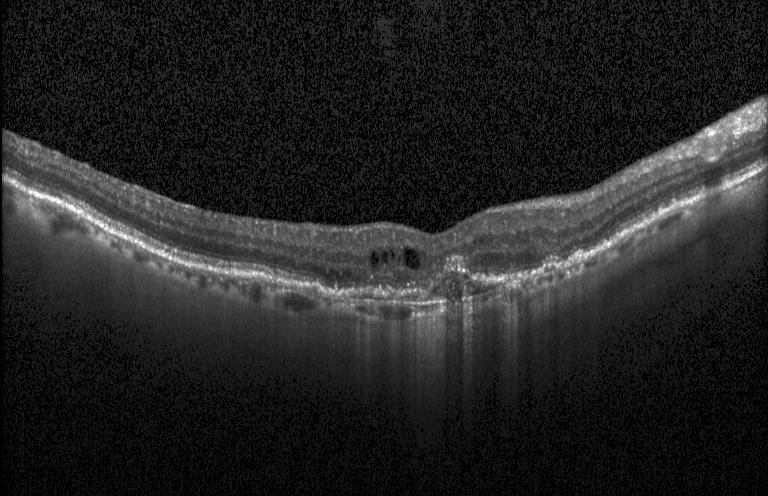

Retinal OCT cross-section showing CNV.